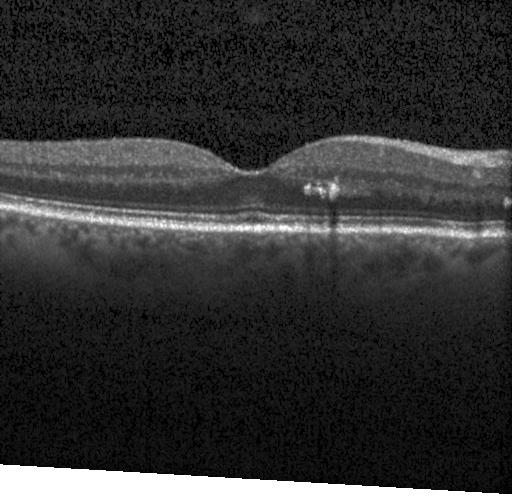 Macular scan · OCT line scan.
This B-scan demonstrates no evidence of choroidal neovascularization, diabetic macular edema, or drusen.